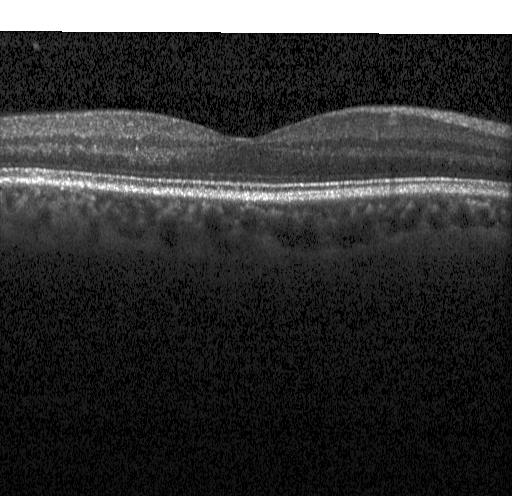

This B-scan demonstrates no CNV, DME, or drusen.